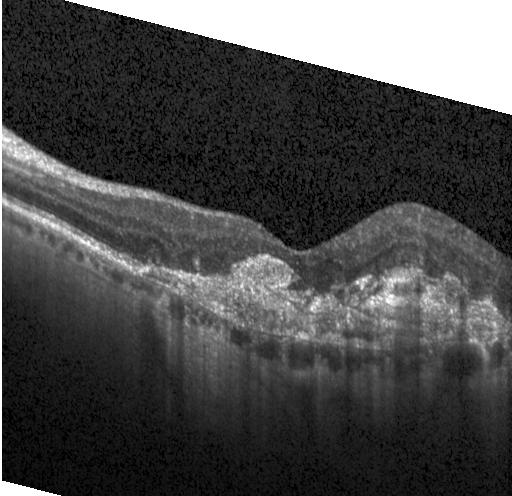 The scan shows CNV.